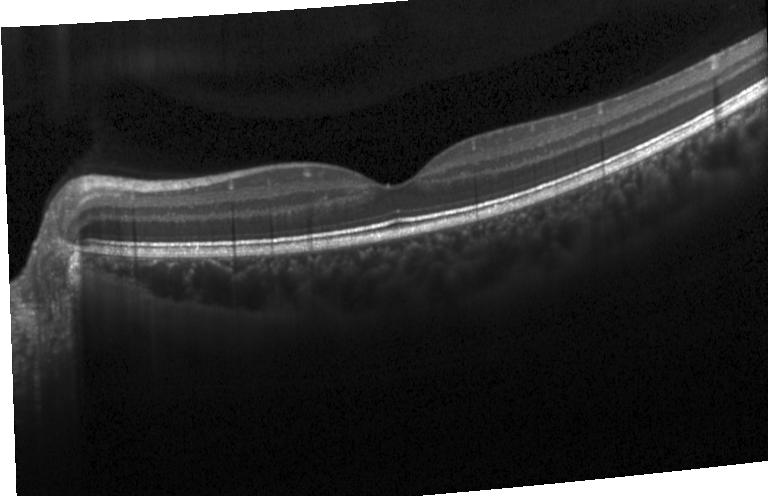
Retinal OCT B-scan. Diagnosis: neither choroidal neovascularization, diabetic macular edema, nor drusen.